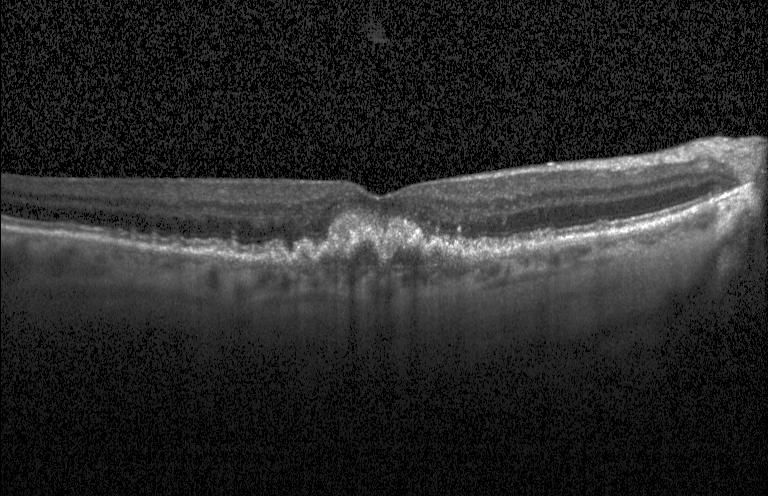
Macular OCT demonstrating a choroidal neovascular membrane.